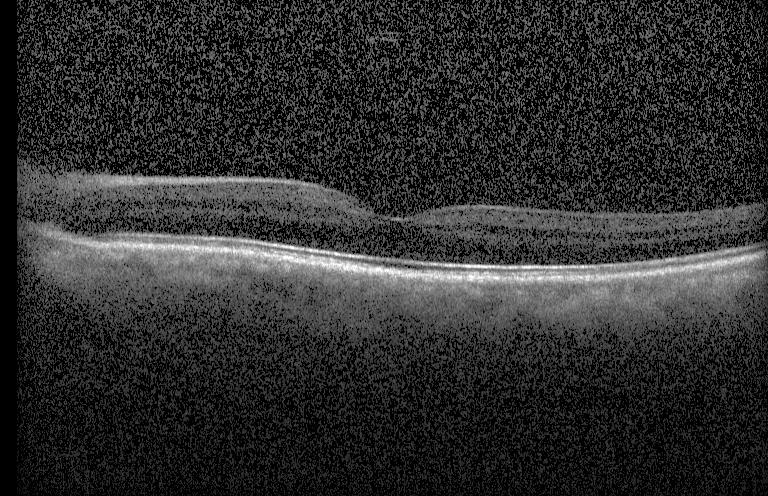 Macular OCT: no evidence of CNV, DME, or drusen.